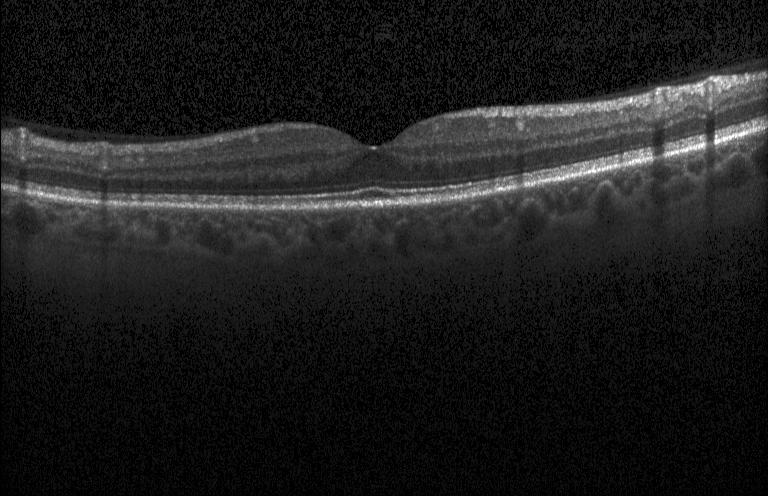 Macular OCT: no evidence of choroidal neovascularization, diabetic macular edema, or drusen.